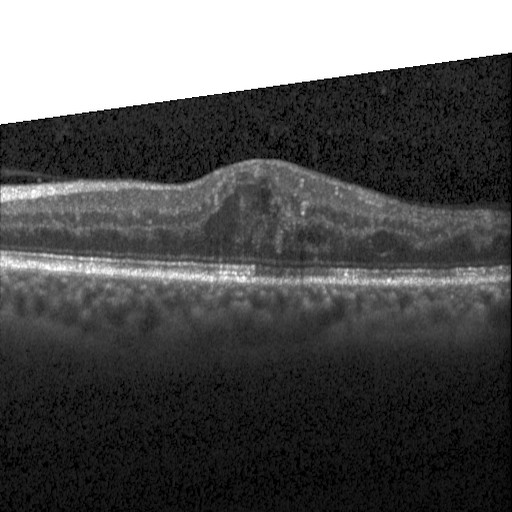
OCT line scan; spectral-domain OCT; acquired on a Heidelberg Spectralis; fovea-centered. Finding: diabetic macular edema (DME).